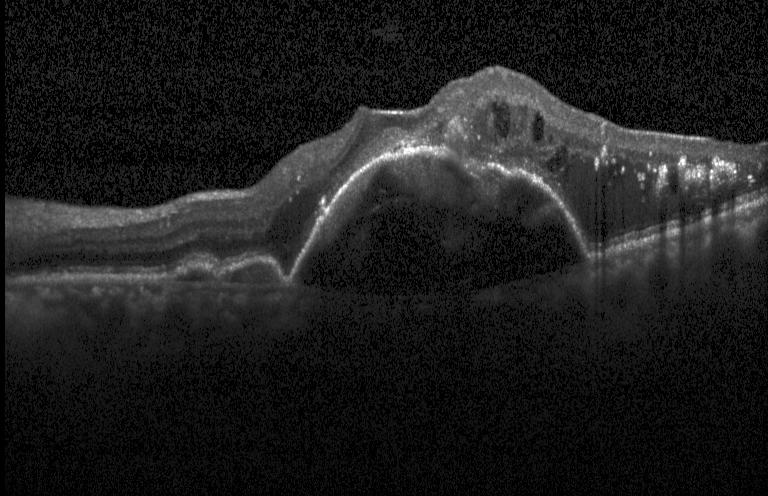

SD-OCT. Optical coherence tomography B-scan. Assessment: a choroidal neovascular membrane.